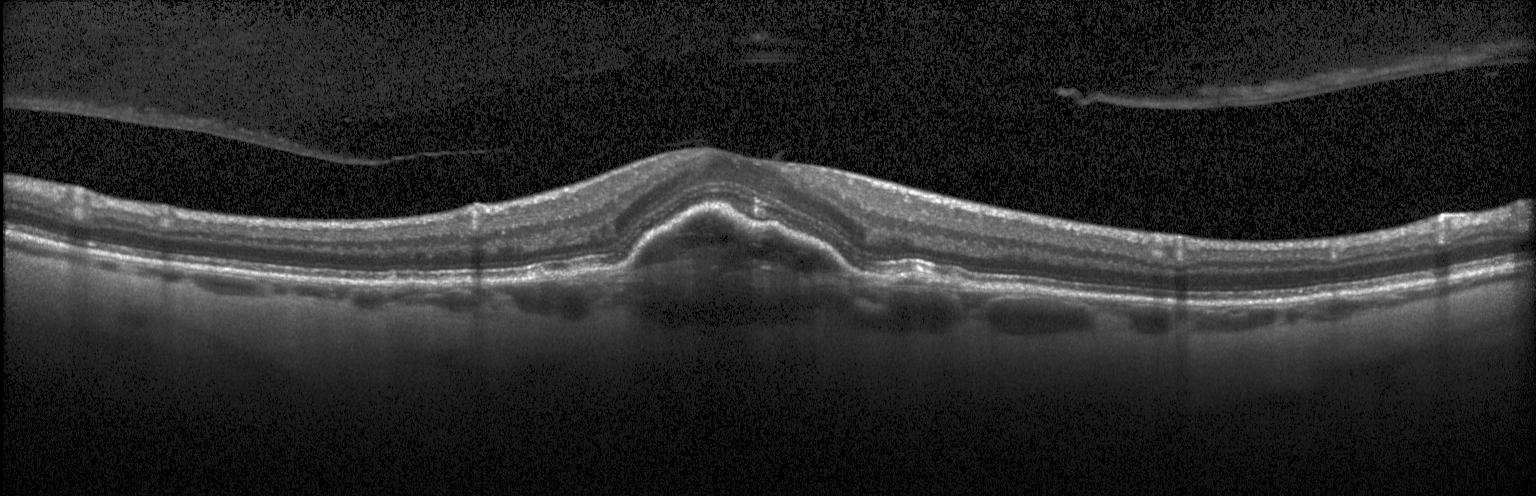
Horizontal scan through the fovea. Retinal OCT cross-section. Spectral-domain optical coherence tomography. Acquired on a Heidelberg Spectralis — The scan shows choroidal neovascularization (CNV).